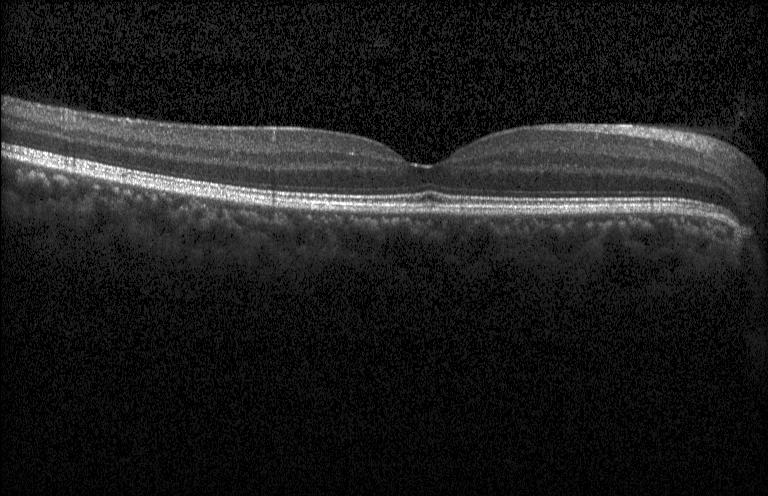
OCT line scan; macular scan.
Impression: no CNV, no DME, and no drusen.